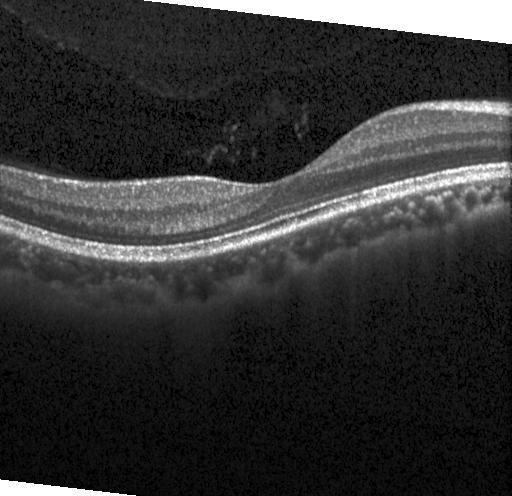 Optical coherence tomography scan
Assessment: no evidence of choroidal neovascularization, diabetic macular edema, or drusen.